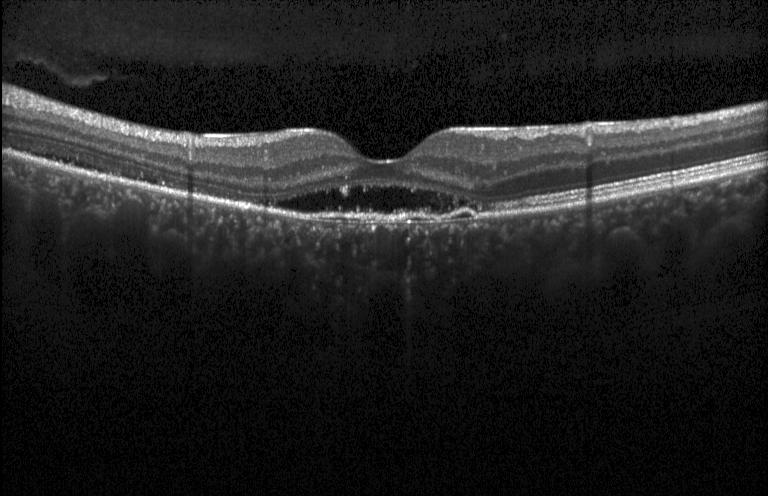 OCT B-scan showing choroidal neovascularization (CNV).